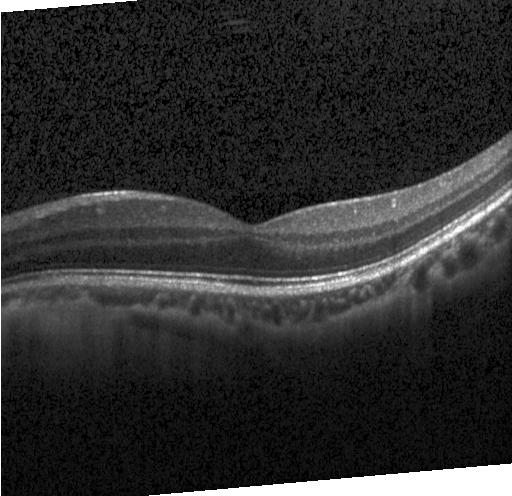 Spectral-domain OCT. Through the macula. Instrument: Heidelberg Spectralis. OCT B-scan. Dx: no evidence of choroidal neovascularization, diabetic macular edema, or drusen.